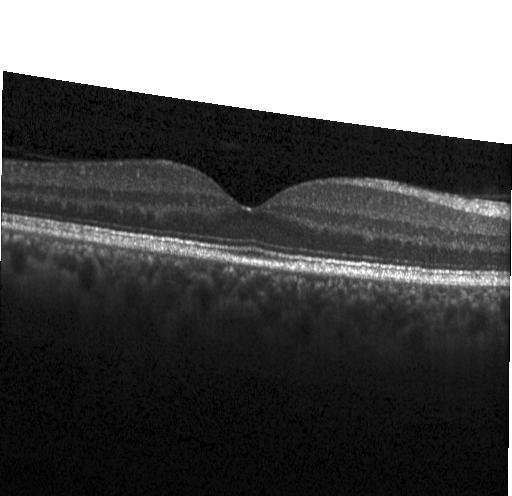 Acquired on a Heidelberg Spectralis, OCT line scan.
Diagnosis: neither choroidal neovascularization, diabetic macular edema, nor drusen.